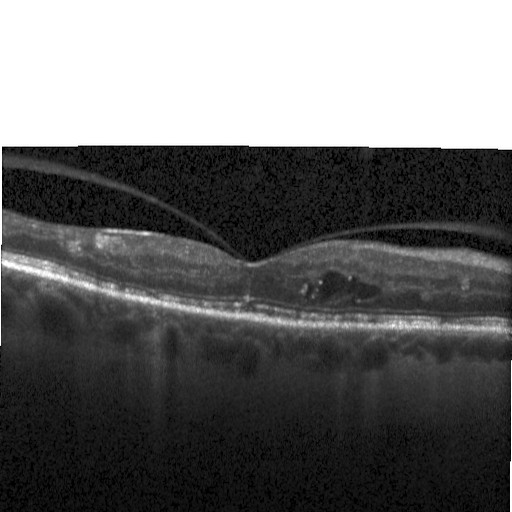 Horizontal scan through the fovea; SD-OCT; retinal OCT B-scan
Assessment: diabetic macular edema.